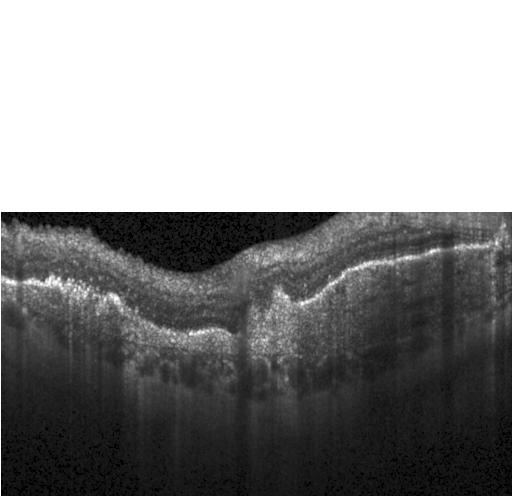 Retinal OCT B-scan; through the macula; Heidelberg Spectralis; spectral-domain OCT. Dx: choroidal neovascularization (CNV).